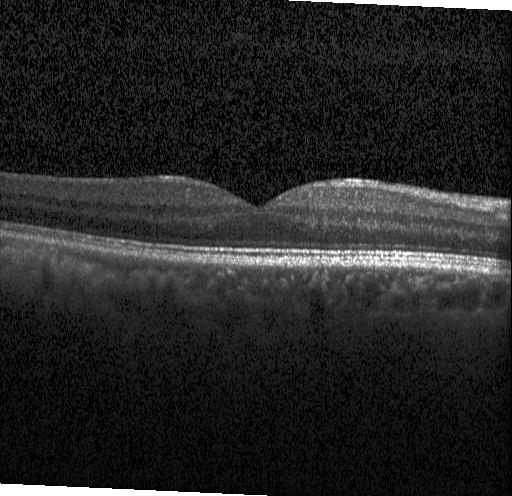

Optical coherence tomography scan.
Finding: no choroidal neovascularization, no diabetic macular edema, and no drusen.